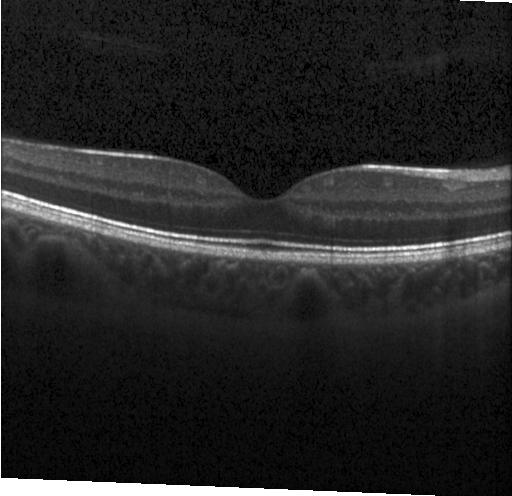
Dx: no choroidal neovascularization, diabetic macular edema, or drusen.